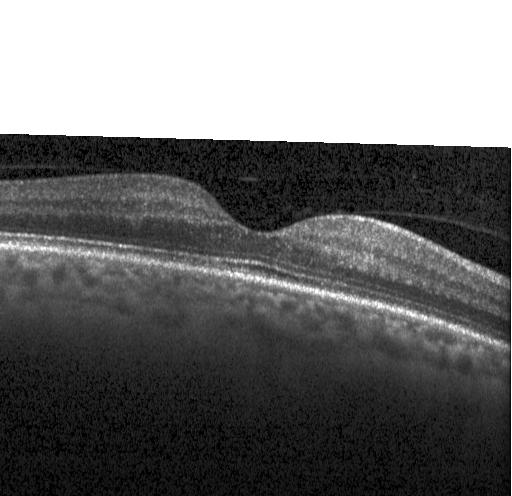
Macular OCT: no choroidal neovascularization, no diabetic macular edema, and no drusen.